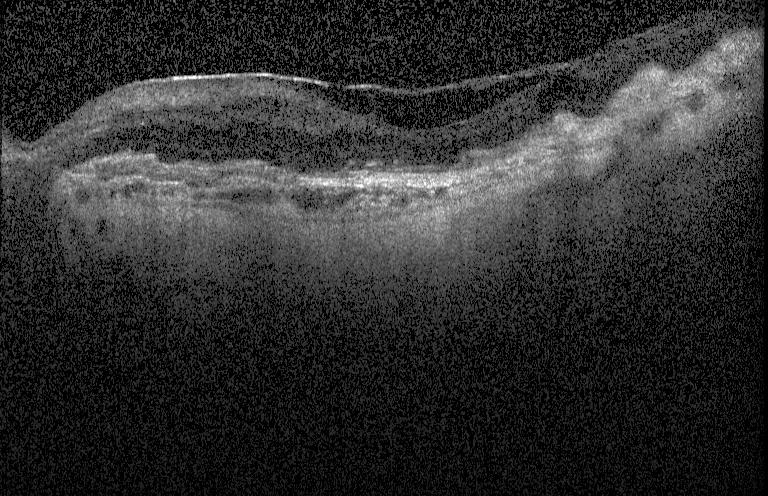 Diagnosis: CNV.